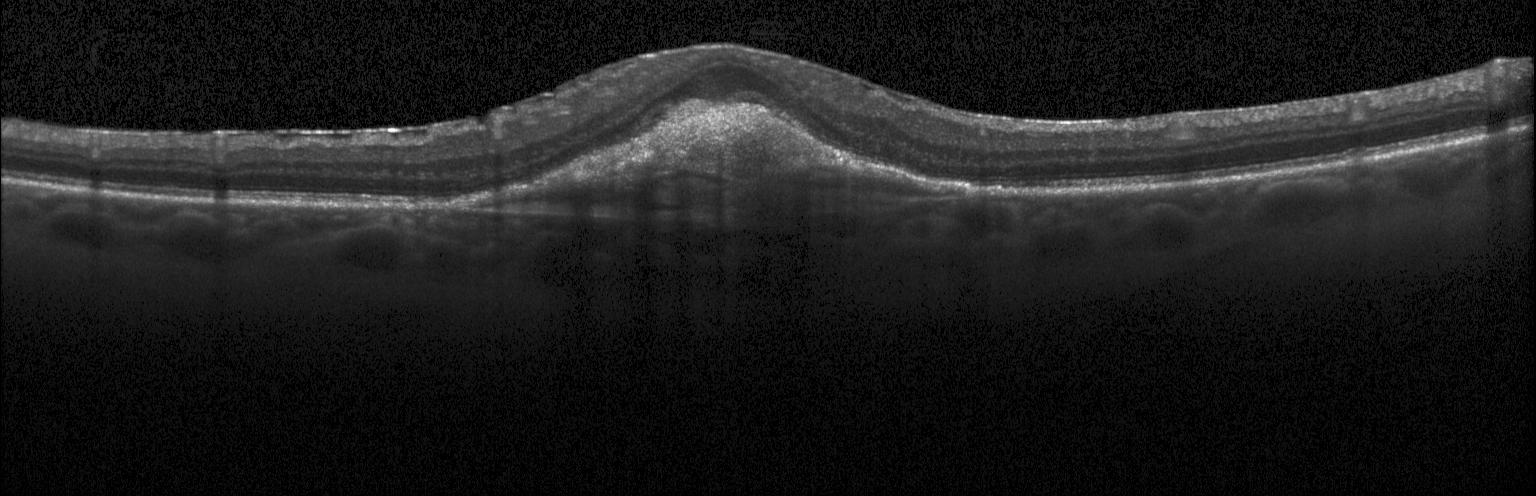 OCT scan showing a choroidal neovascular membrane.